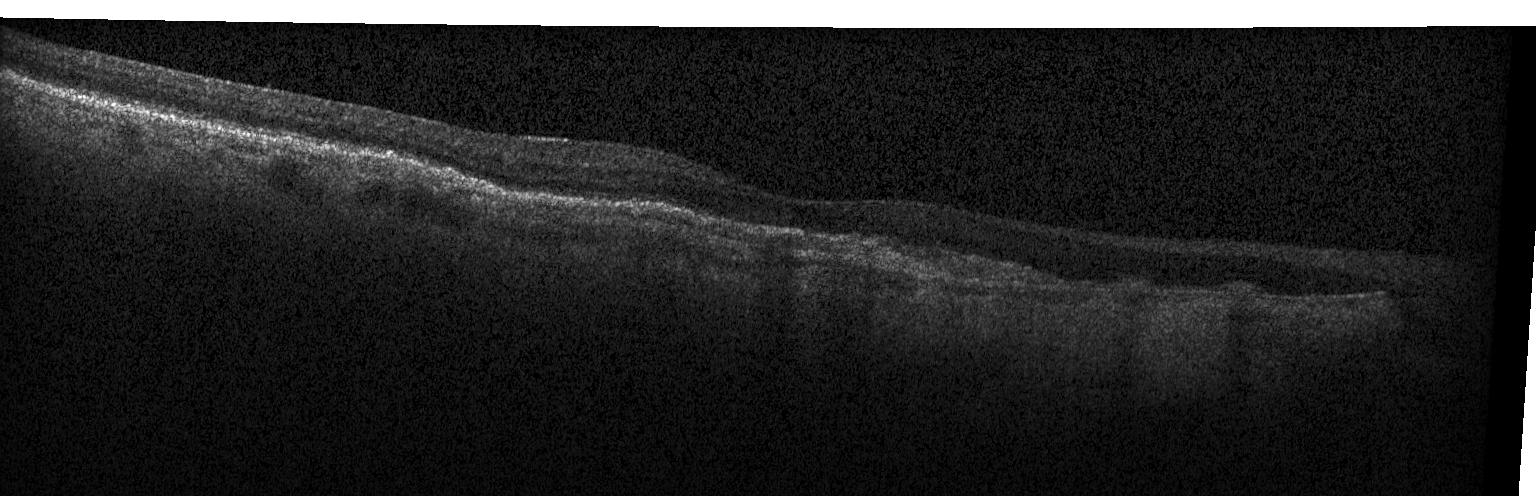
Retinal OCT B-scan
A choroidal neovascular membrane.